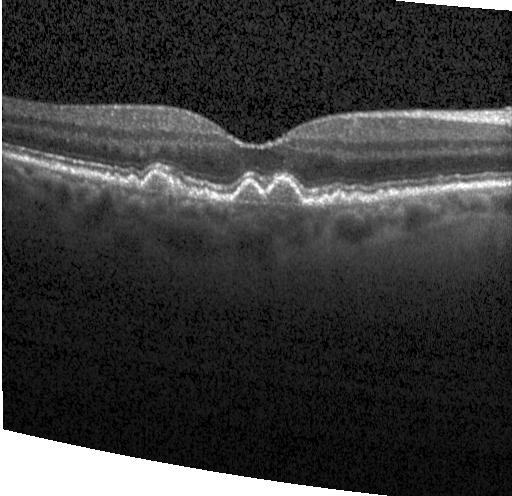 Macular scan · spectral-domain OCT · acquired on a Heidelberg Spectralis · optical coherence tomography scan — This B-scan demonstrates sub-RPE drusenoid deposits.